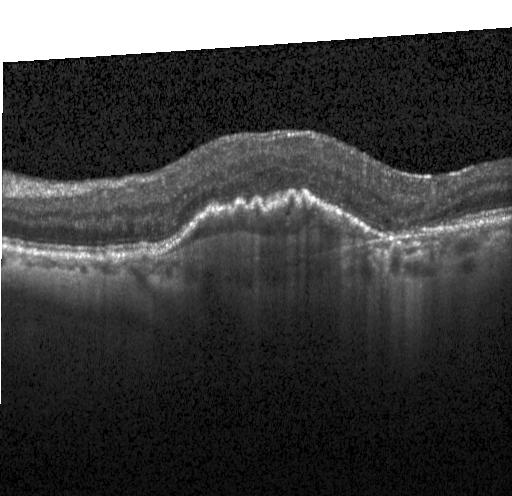 The scan shows a choroidal neovascular membrane.